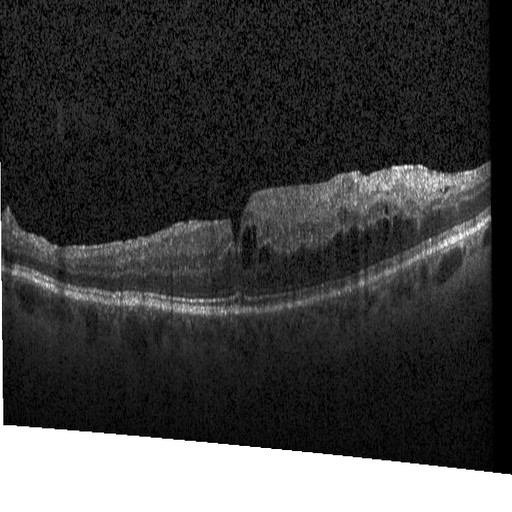
Diabetic macular edema.